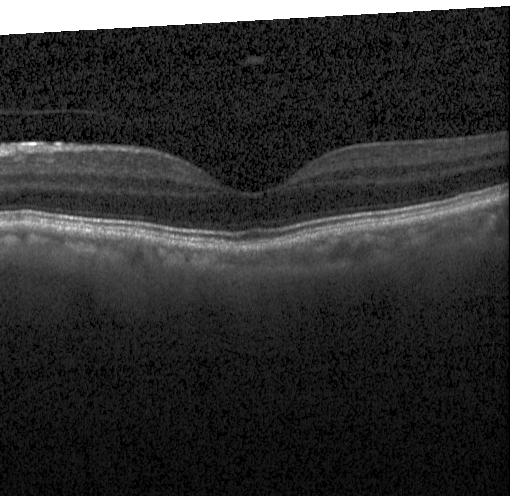 Retinal OCT cross-section, Heidelberg Spectralis OCT system, SD-OCT
The scan shows neither choroidal neovascularization, diabetic macular edema, nor drusen.